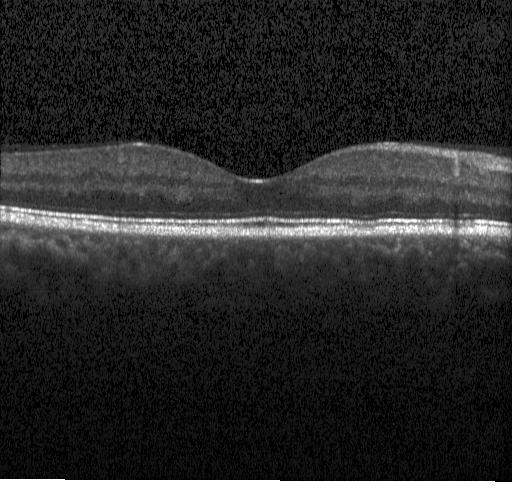

Acquired on a Heidelberg Spectralis; spectral-domain optical coherence tomography; OCT B-scan
OCT finding: no choroidal neovascularization, diabetic macular edema, or drusen.